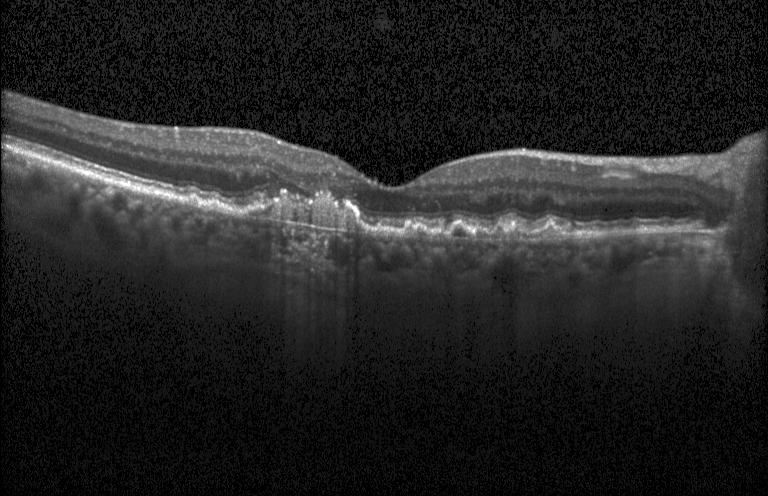 OCT B-scan showing a choroidal neovascular membrane.